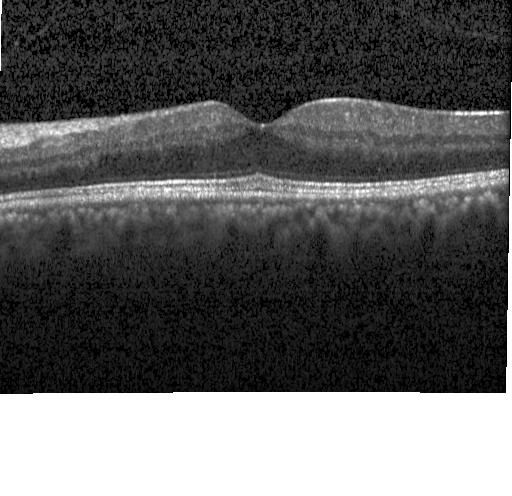

OCT line scan, instrument: Heidelberg Spectralis, fovea-centered
No evidence of choroidal neovascularization, diabetic macular edema, or drusen.